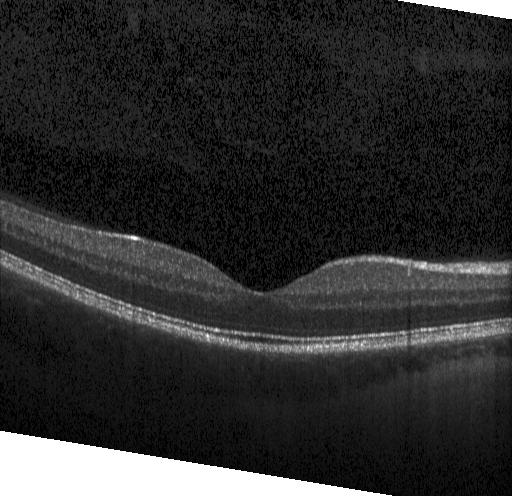 Finding: no choroidal neovascularization, no diabetic macular edema, and no drusen.